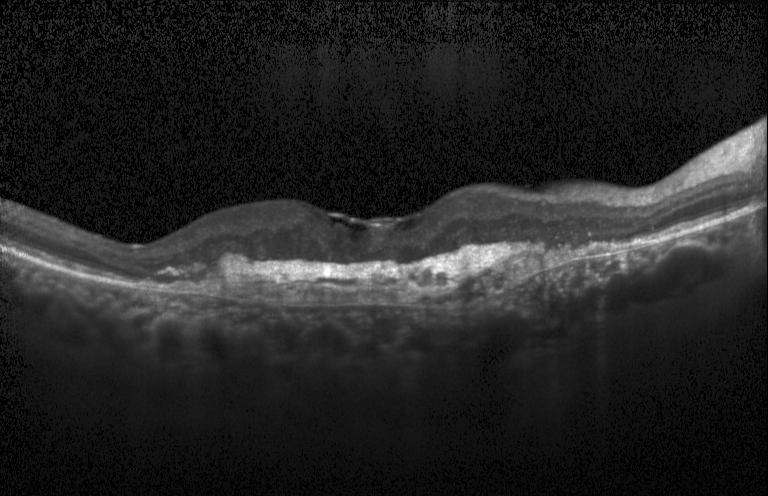
Dx: CNV.